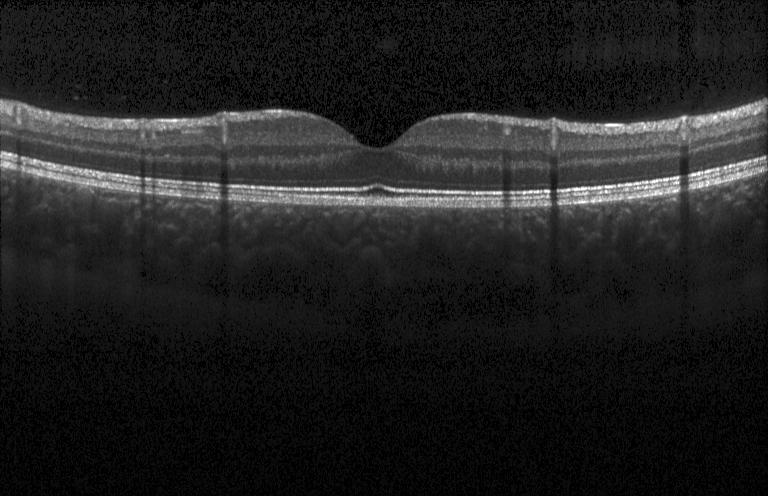
Spectral-domain OCT, optical coherence tomography B-scan.
Impression: no choroidal neovascularization, no diabetic macular edema, and no drusen.